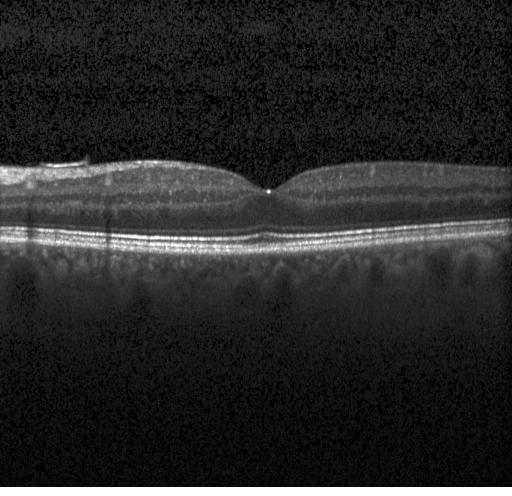

Instrument: Heidelberg Spectralis; retinal OCT cross-section; SD-OCT — The scan shows no choroidal neovascularization, diabetic macular edema, or drusen.